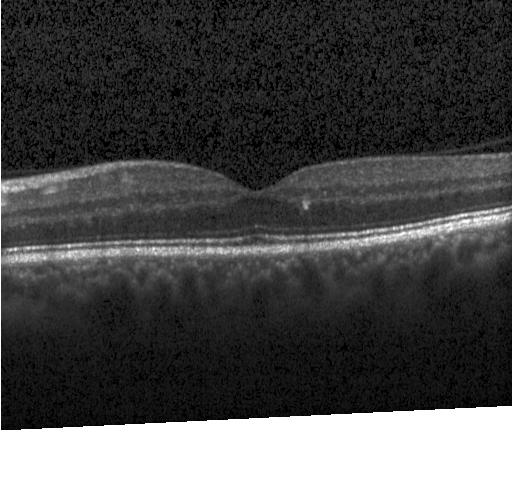 Impression: no evidence of CNV, DME, or drusen.